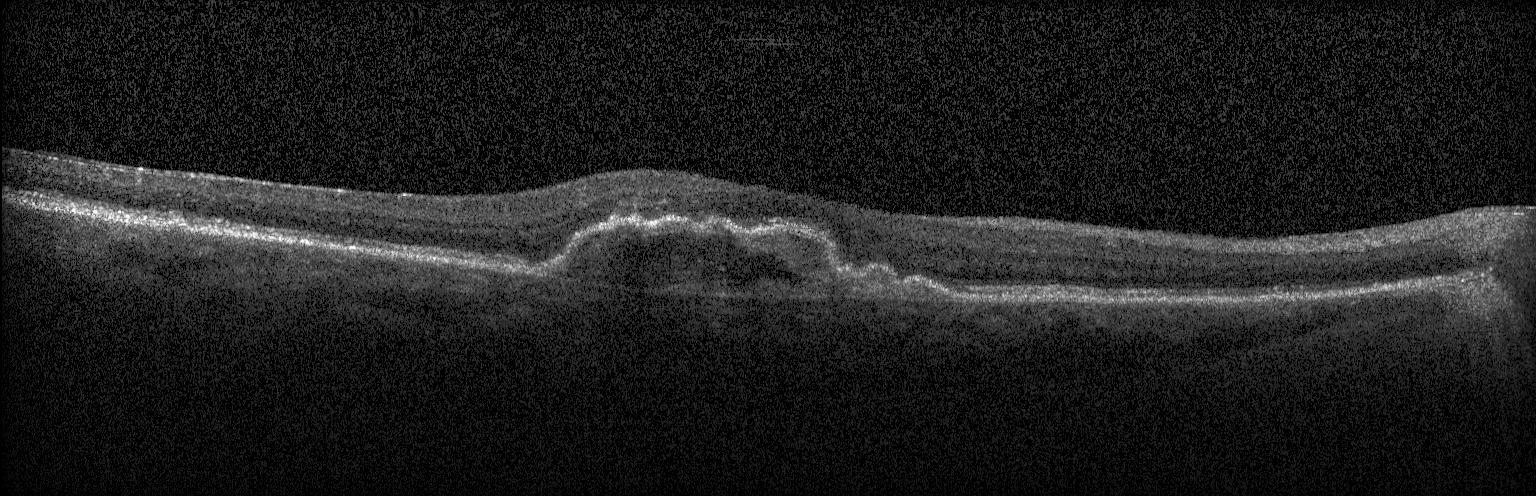

Acquired on a Heidelberg Spectralis. Optical coherence tomography scan. Through the macula
Macular OCT: CNV.